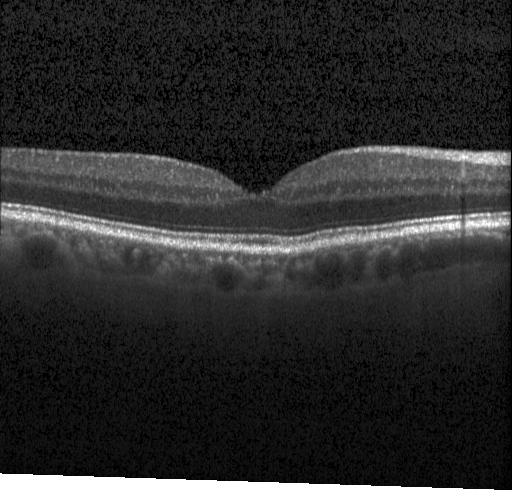
Spectral-domain OCT B-scan: no choroidal neovascularization, no diabetic macular edema, and no drusen.